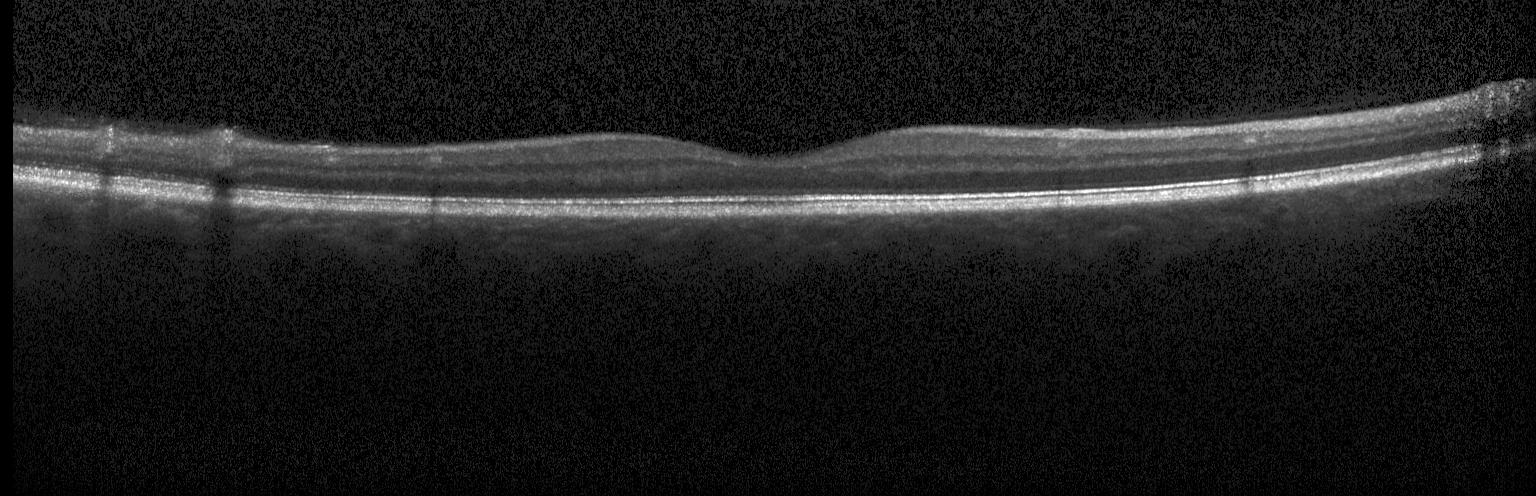
Neither CNV, DME, nor drusen.